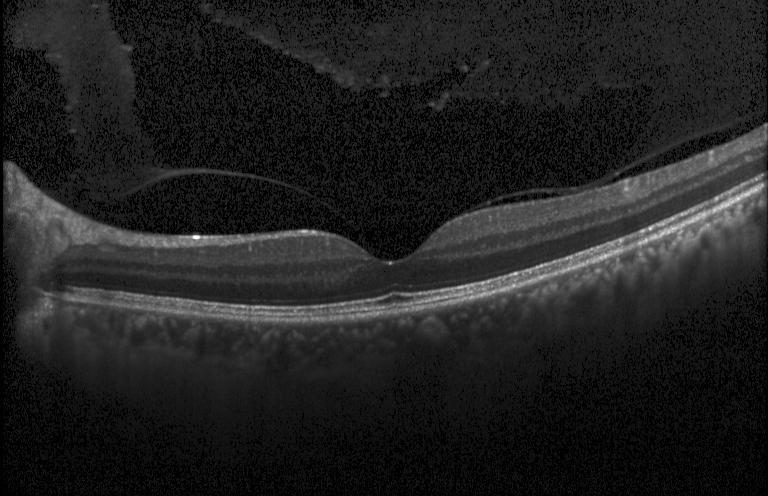 Spectral-domain OCT. Retinal OCT cross-section.
The scan shows no evidence of choroidal neovascularization, diabetic macular edema, or drusen.